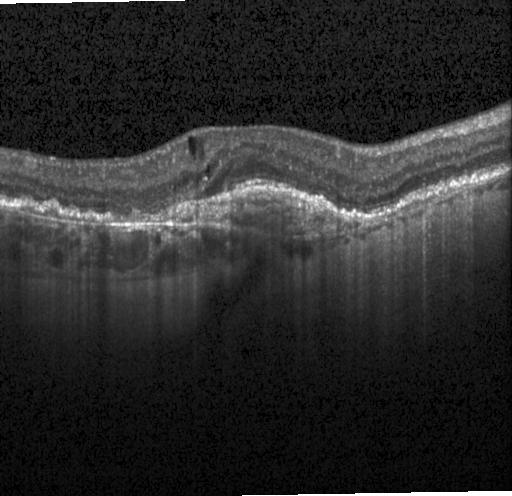 The scan shows choroidal neovascularization.